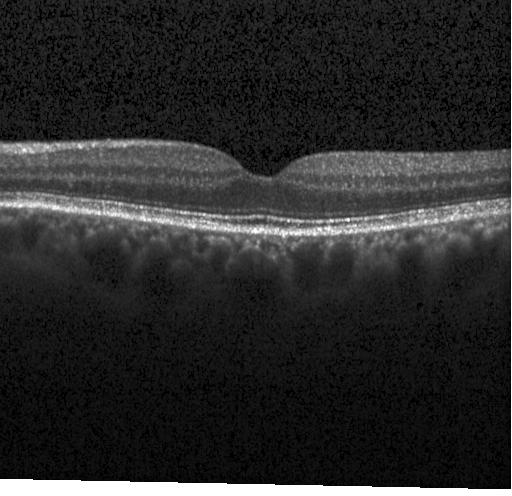 SD-OCT · optical coherence tomography B-scan
Impression: neither CNV, DME, nor drusen.